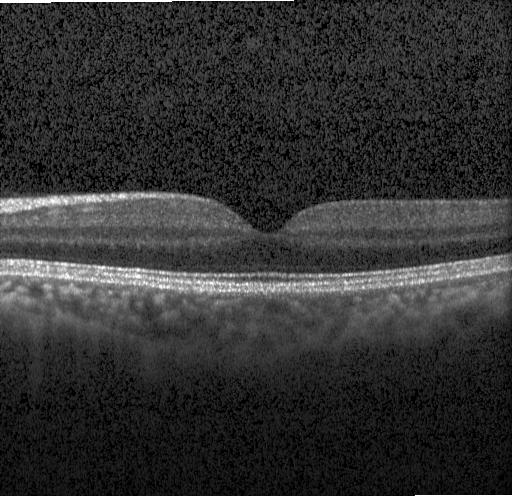 No evidence of choroidal neovascularization, diabetic macular edema, or drusen.